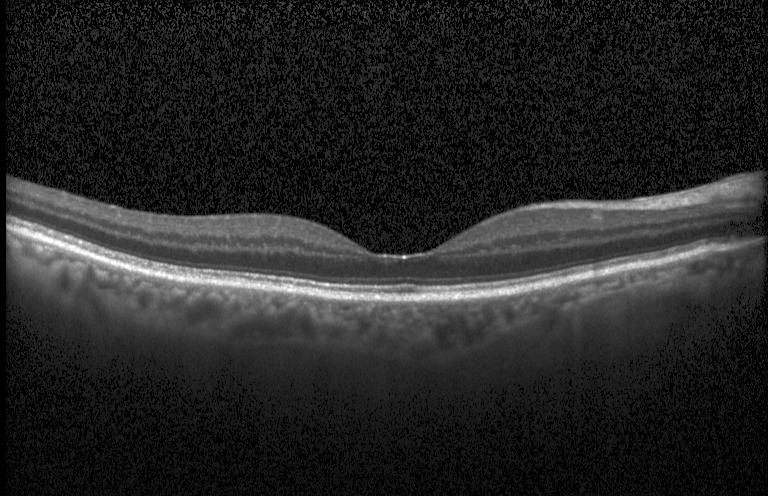
Diagnosis: no CNV, DME, or drusen.